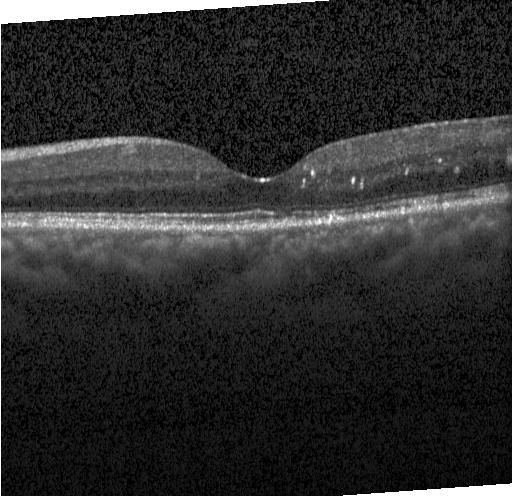
Macular scan. Acquired on a Heidelberg Spectralis. Optical coherence tomography B-scan. SD-OCT
OCT finding: diabetic macular edema.